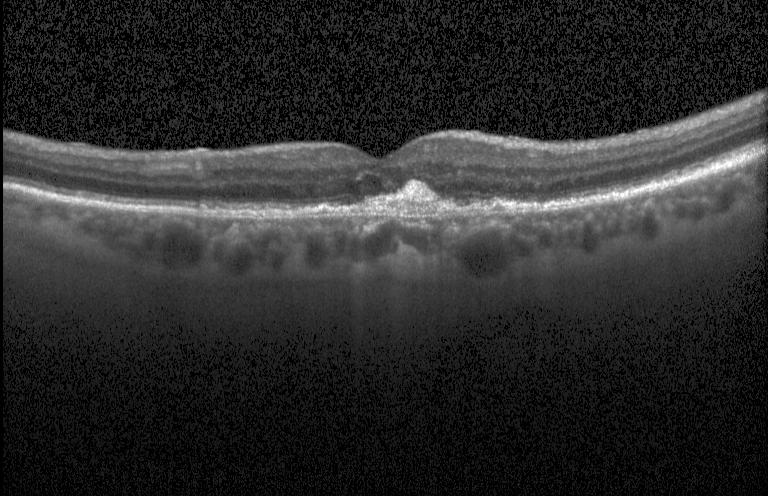 Retinal OCT B-scan, Heidelberg Spectralis — Macular OCT: choroidal neovascularization (CNV).